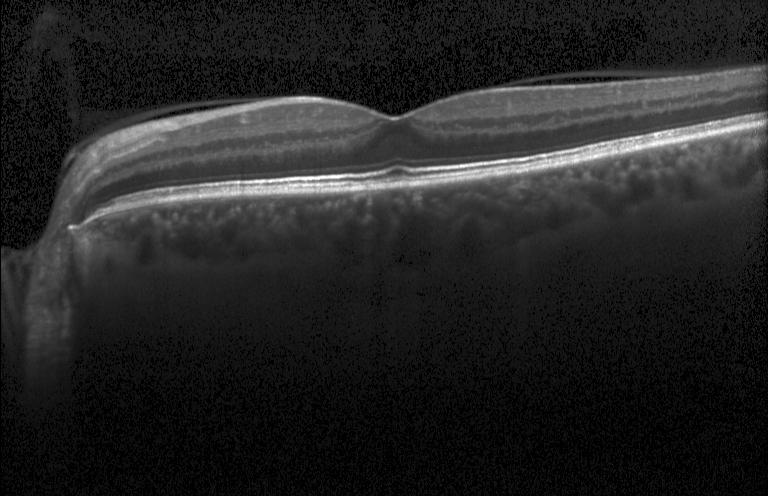
Optical coherence tomography scan. The scan shows no evidence of CNV, DME, or drusen.